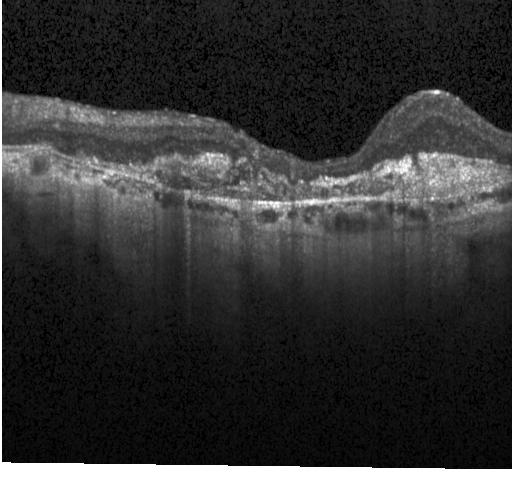 The scan shows a choroidal neovascular membrane.